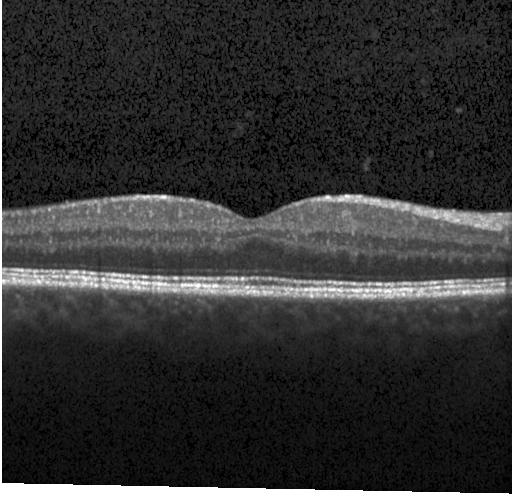 Impression: neither choroidal neovascularization, diabetic macular edema, nor drusen.